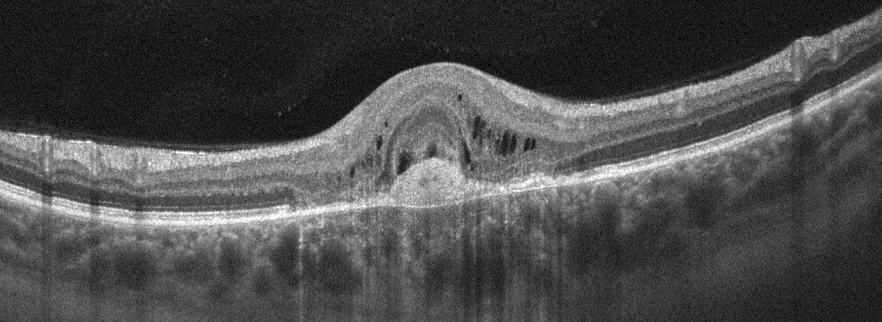

Optical coherence tomography B-scan
Impression: age-related macular degeneration.